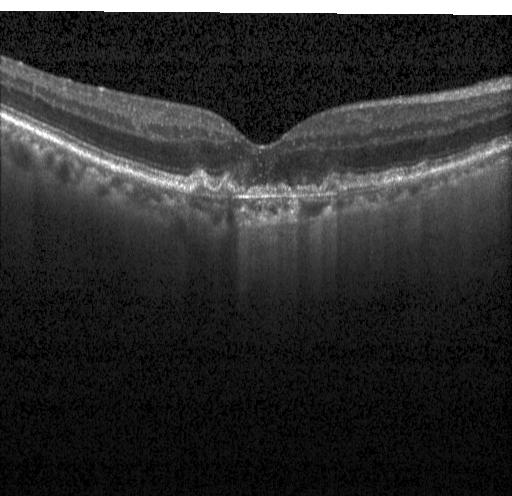

Spectral-domain optical coherence tomography · horizontal scan through the fovea · optical coherence tomography scan · instrument: Heidelberg Spectralis.
Impression: drusen.